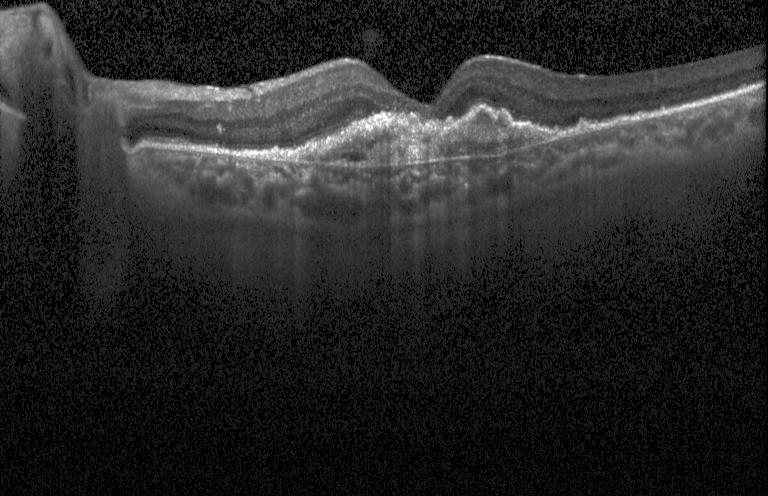 Optical coherence tomography scan — OCT finding: a choroidal neovascular membrane.